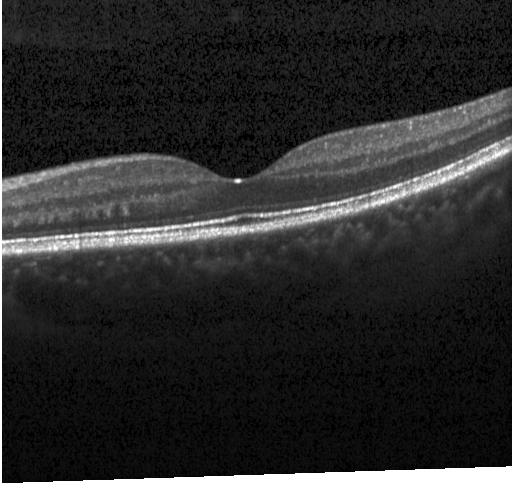 Fovea-centered; spectral-domain OCT; retinal OCT B-scan.
Macular OCT: no choroidal neovascularization, diabetic macular edema, or drusen.